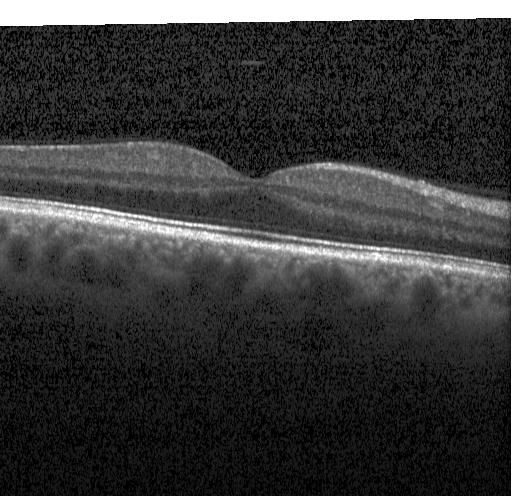

Impression: no choroidal neovascularization, diabetic macular edema, or drusen.